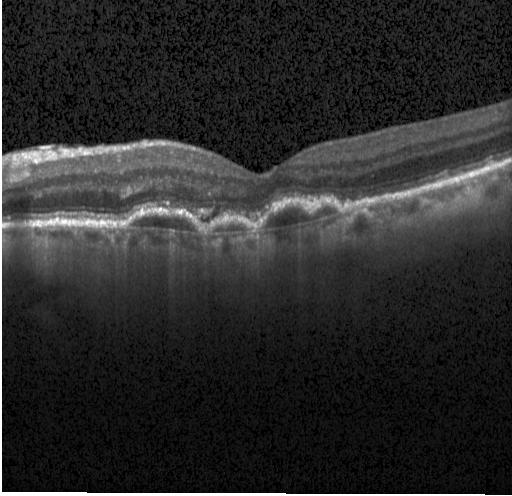
Spectral-domain OCT B-scan: a choroidal neovascular membrane.